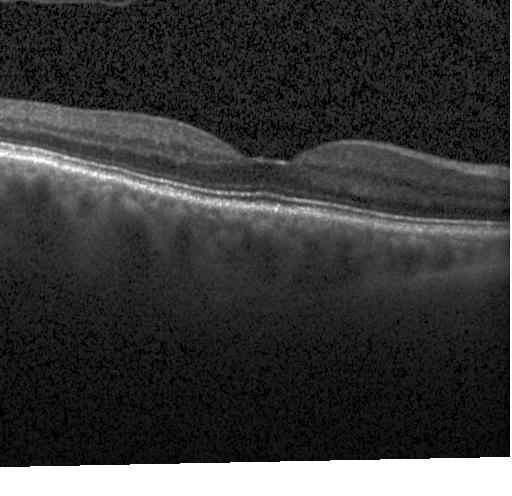

Finding: no evidence of choroidal neovascularization, diabetic macular edema, or drusen.